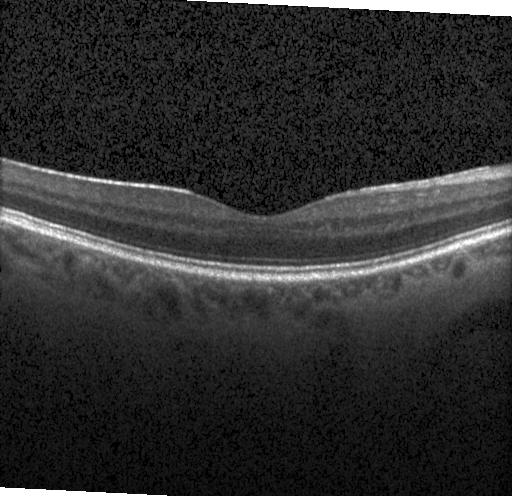 Fovea-centered, instrument: Heidelberg Spectralis, optical coherence tomography B-scan — Diagnosis: no CNV, no DME, and no drusen.